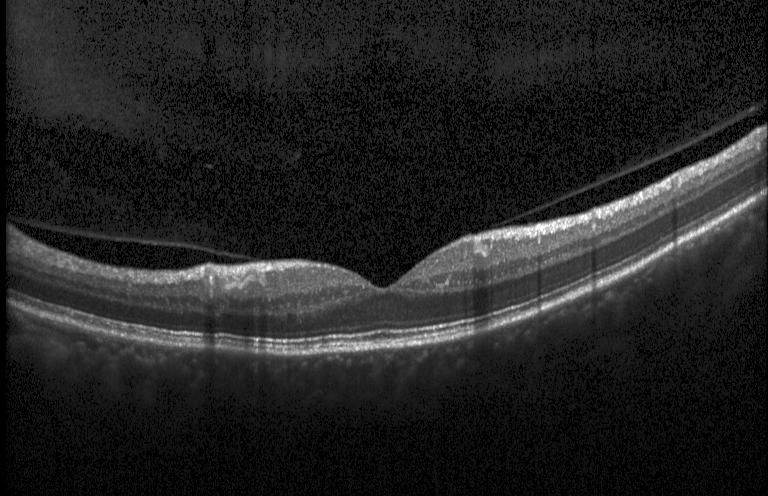
Macular scan · retinal OCT cross-section · instrument: Heidelberg Spectralis · SD-OCT — Diagnosis: no evidence of choroidal neovascularization, diabetic macular edema, or drusen.